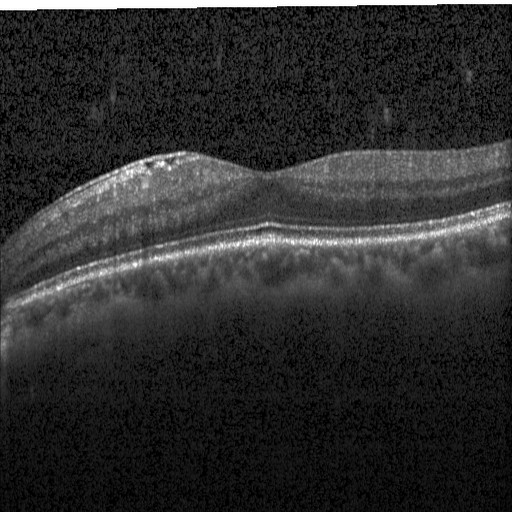
Optical coherence tomography scan. Diabetic macular edema.